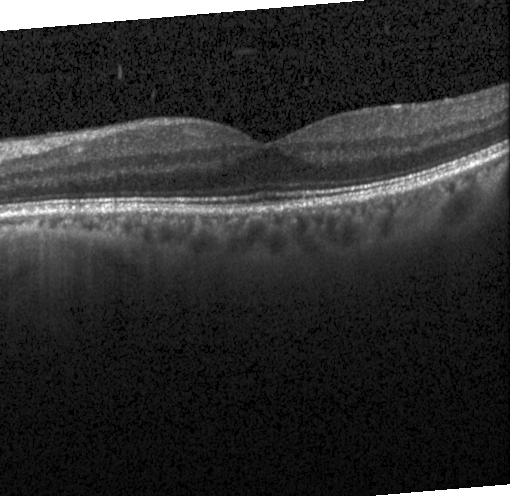 OCT line scan · spectral-domain OCT · centered on the fovea — Neither CNV, DME, nor drusen.